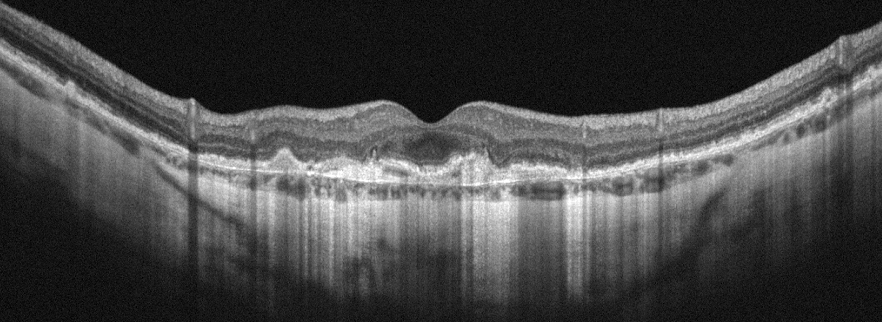

Optical coherence tomography scan · oculus dexter. Dx: age-related macular degeneration (AMD).